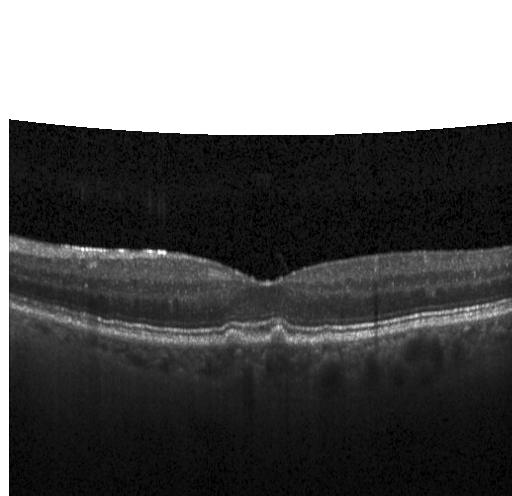
Spectral-domain OCT; OCT B-scan — Impression: drusen.